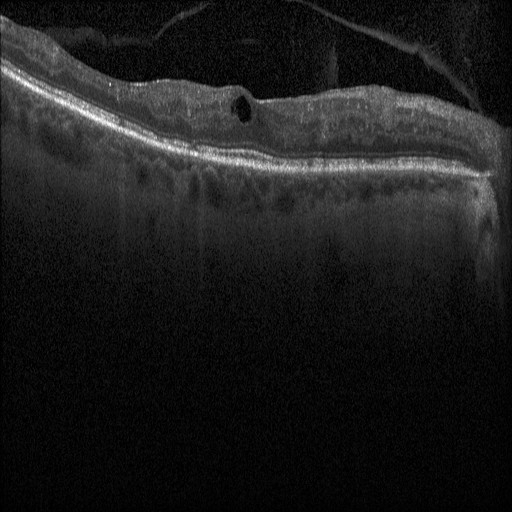
Macular OCT: diabetic macular edema (DME).